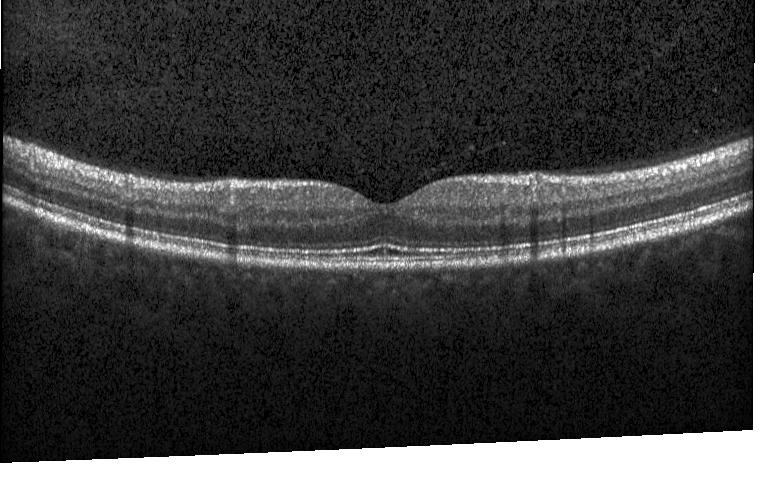 This B-scan demonstrates neither choroidal neovascularization, diabetic macular edema, nor drusen.